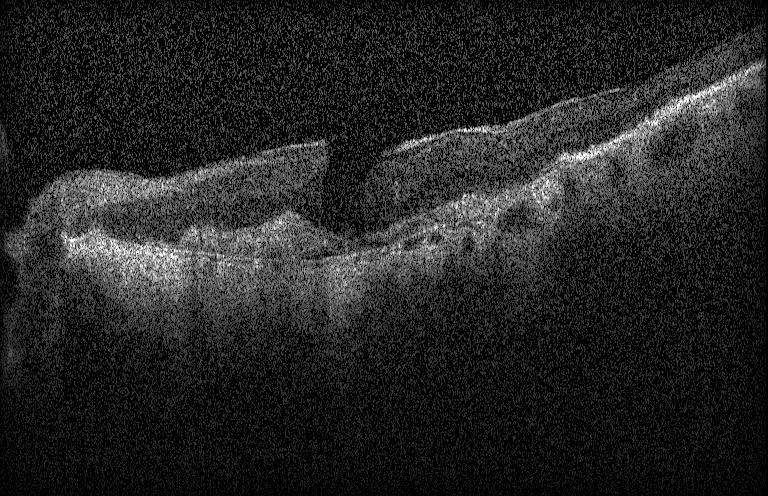
Instrument: Heidelberg Spectralis, retinal OCT B-scan, fovea-centered. Assessment: a choroidal neovascular membrane.